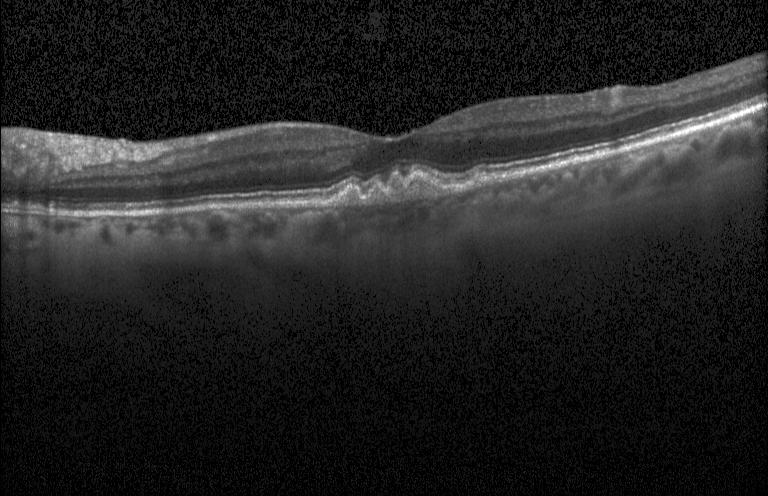
Retinal OCT cross-section showing multiple drusen.